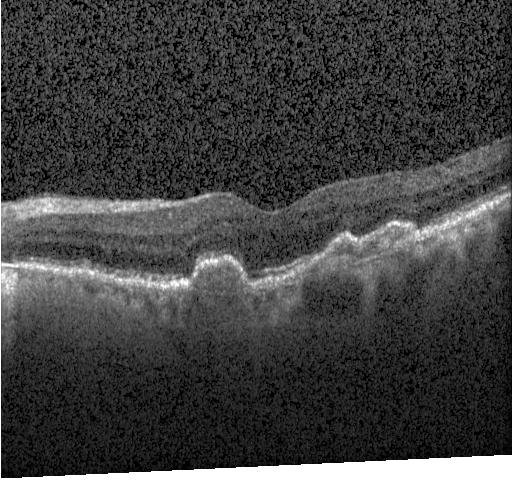 Acquired on a Heidelberg Spectralis. Retinal OCT B-scan. Impression: a choroidal neovascular membrane.